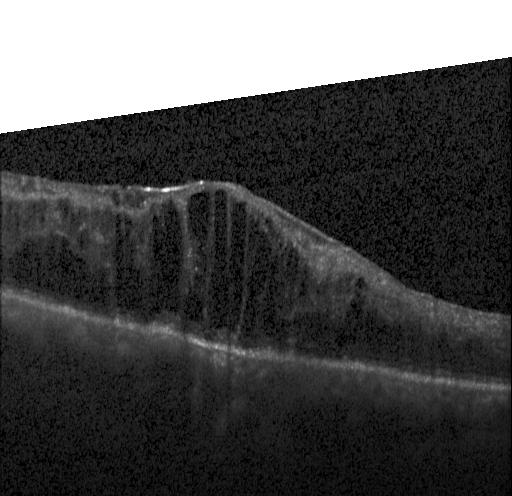
Macular OCT: diabetic macular edema (DME).